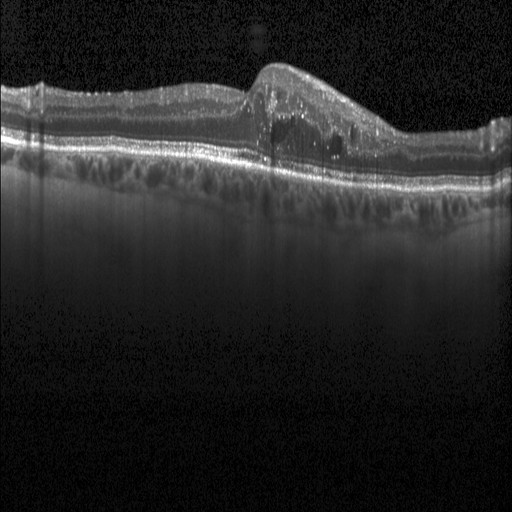
SD-OCT · Heidelberg Spectralis OCT system · optical coherence tomography B-scan · fovea-centered.
Diagnosis: diabetic macular edema.